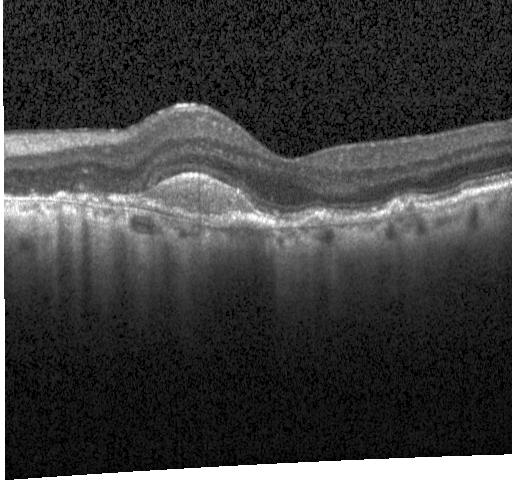
Macular scan. OCT line scan. Spectral-domain optical coherence tomography. Acquired on a Heidelberg Spectralis.
Macular OCT: choroidal neovascularization.